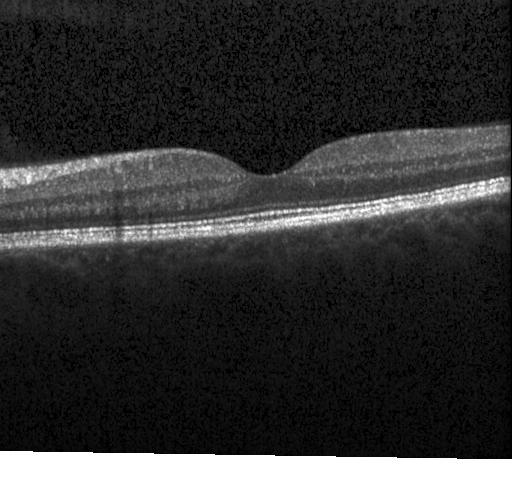
OCT line scan; instrument: Heidelberg Spectralis. Diagnosis: no CNV, DME, or drusen.